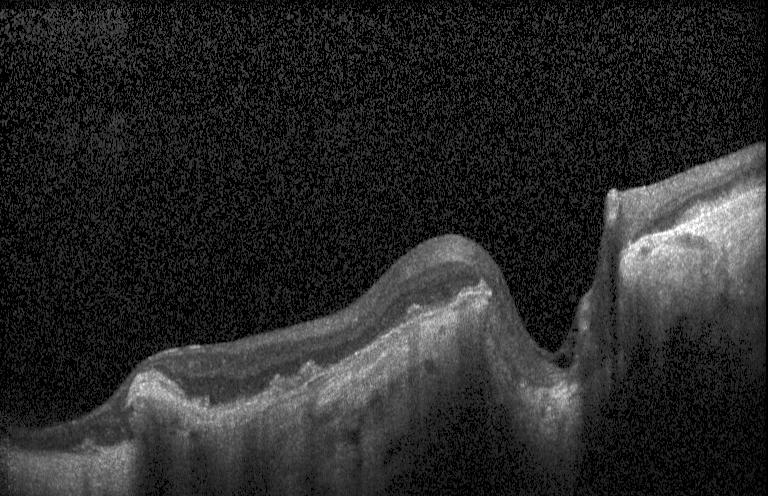 Diagnosis: CNV.